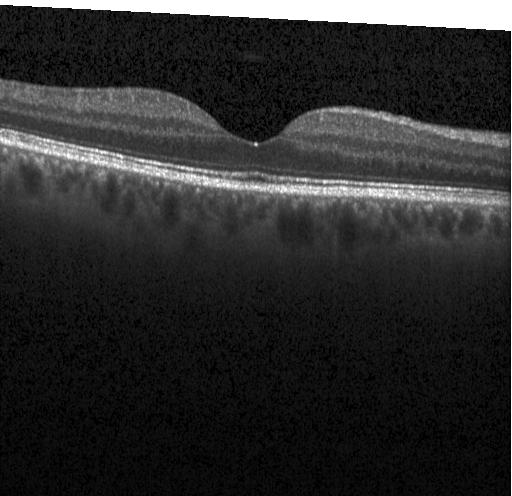 Macular OCT: no choroidal neovascularization, no diabetic macular edema, and no drusen.